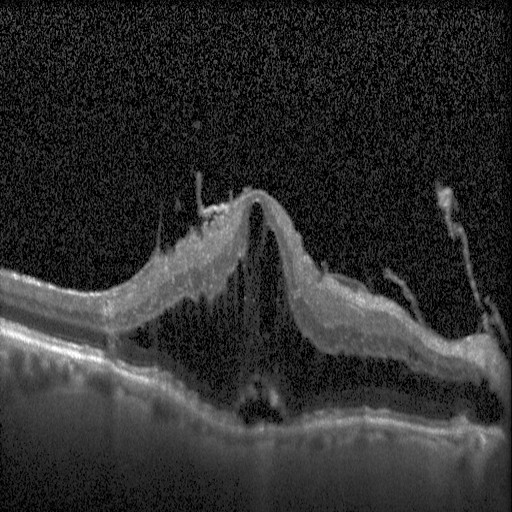
Diabetic macular edema.